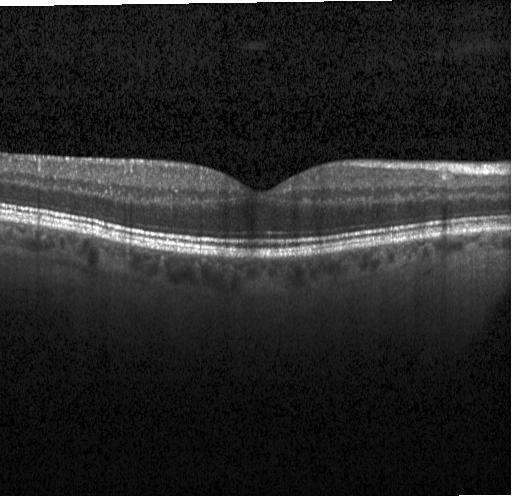
Optical coherence tomography scan — Diagnosis: no choroidal neovascularization, diabetic macular edema, or drusen.